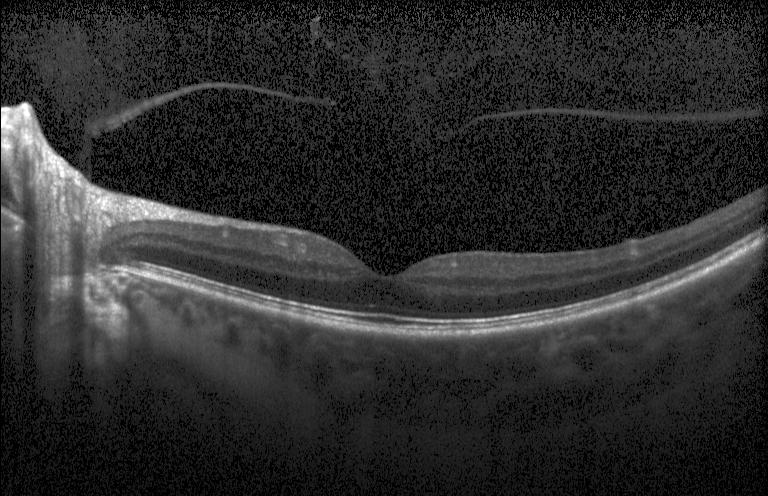

Finding: neither choroidal neovascularization, diabetic macular edema, nor drusen.